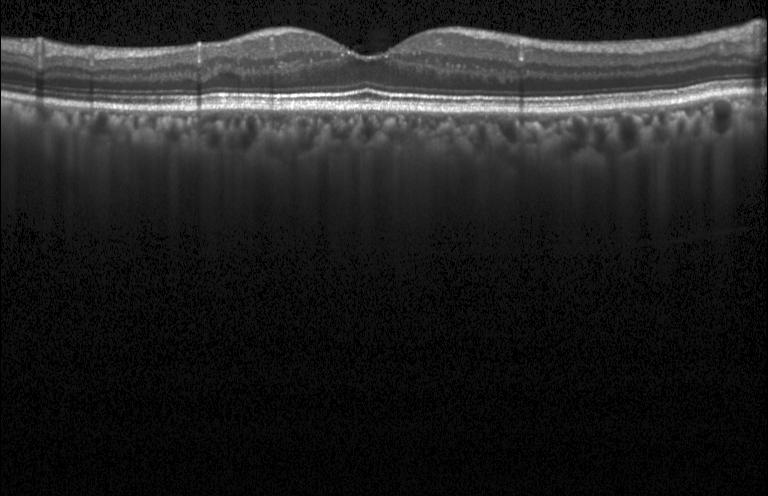

Retinal OCT B-scan. Through the macula. Spectral-domain optical coherence tomography
Dx: neither choroidal neovascularization, diabetic macular edema, nor drusen.